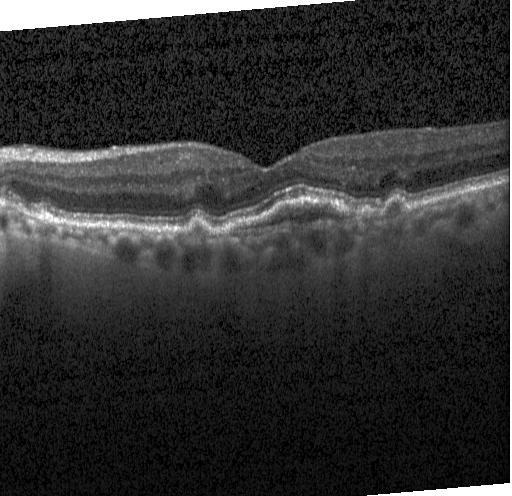
Diagnosis: a choroidal neovascular membrane.